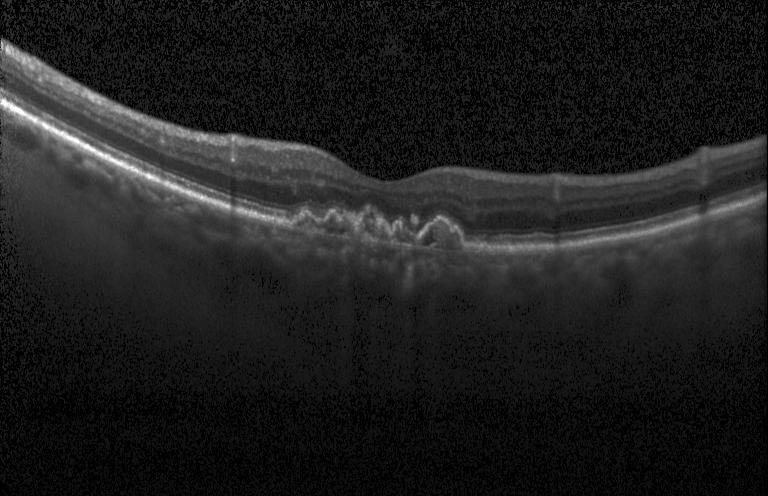 Optical coherence tomography scan, macular scan
Finding: CNV.